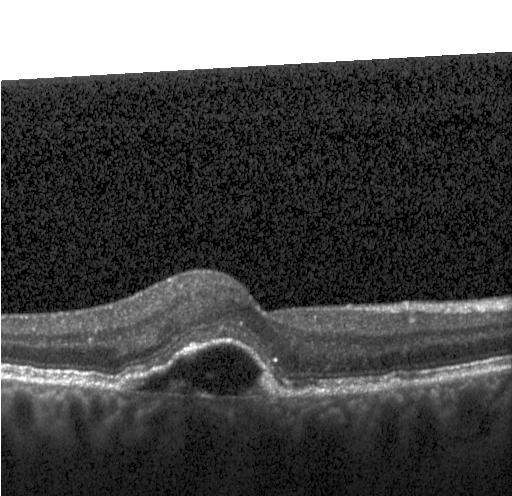

Spectral-domain OCT. Retinal OCT B-scan — Finding: a choroidal neovascular membrane.